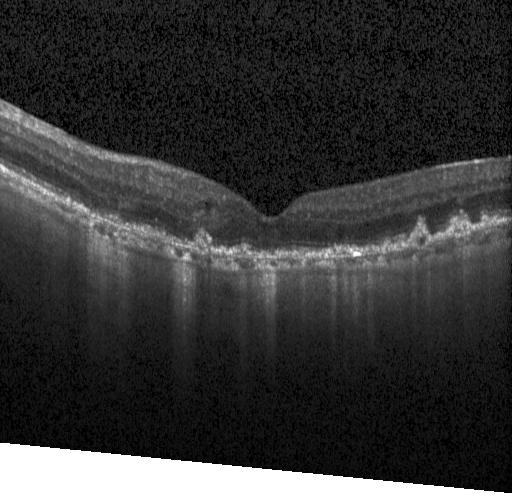 Diagnosis: CNV.